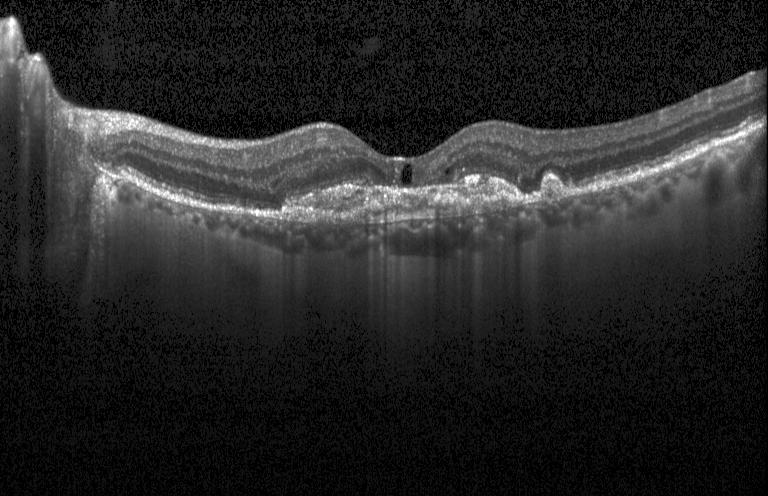
Optical coherence tomography B-scan, acquired on a Heidelberg Spectralis — Finding: a choroidal neovascular membrane.